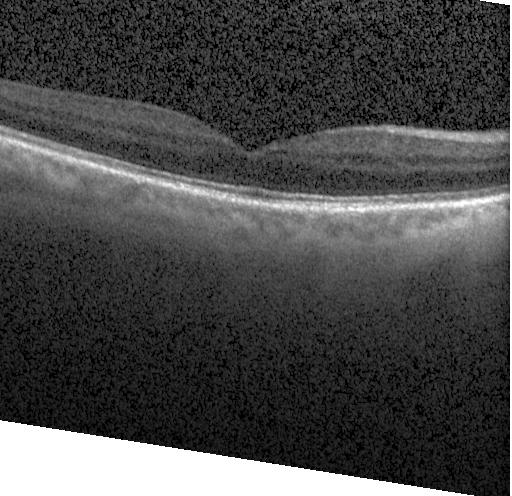

Macular OCT demonstrating no choroidal neovascularization, diabetic macular edema, or drusen.